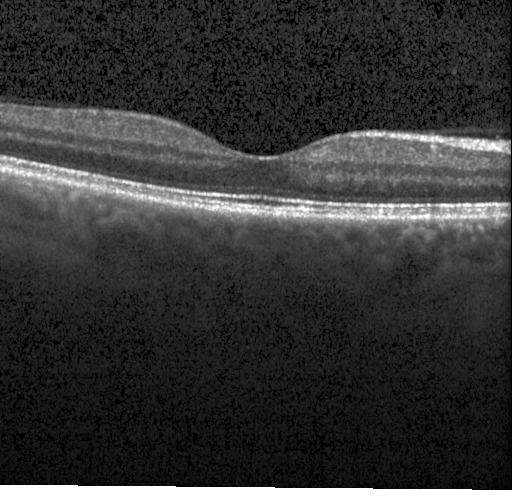
OCT B-scan. The scan shows no choroidal neovascularization, no diabetic macular edema, and no drusen.